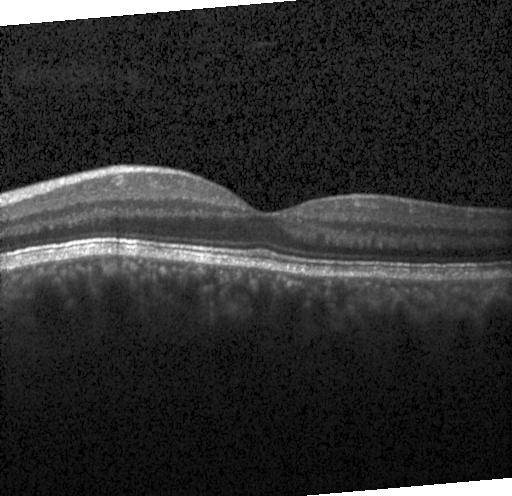 Optical coherence tomography scan. Heidelberg Spectralis. SD-OCT — Dx: neither choroidal neovascularization, diabetic macular edema, nor drusen.